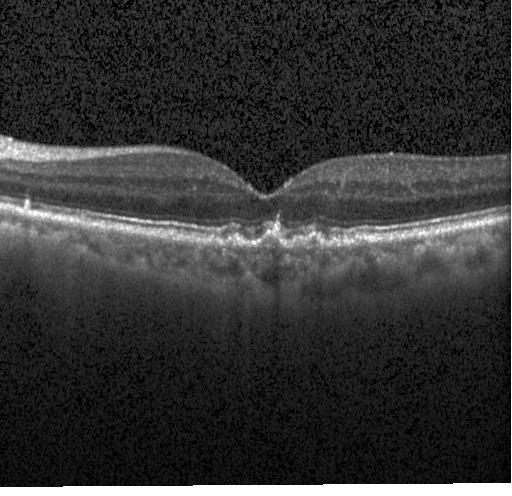

Retinal OCT B-scan; Heidelberg Spectralis — The scan shows multiple drusen.